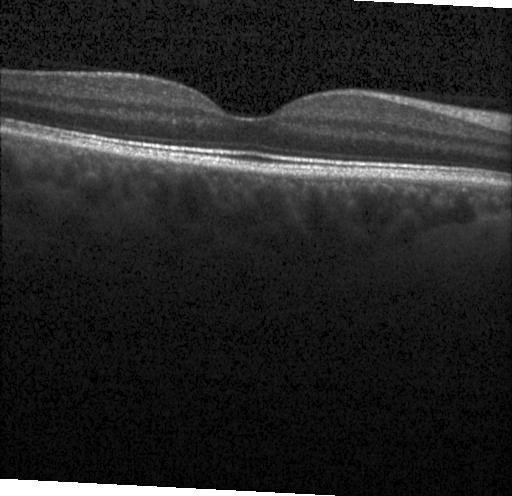

Macular scan, OCT line scan. Finding: no choroidal neovascularization, diabetic macular edema, or drusen.